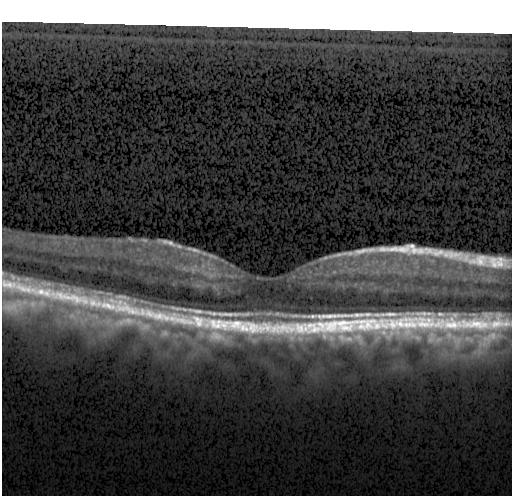
Optical coherence tomography scan
Diagnosis: no CNV, no DME, and no drusen.